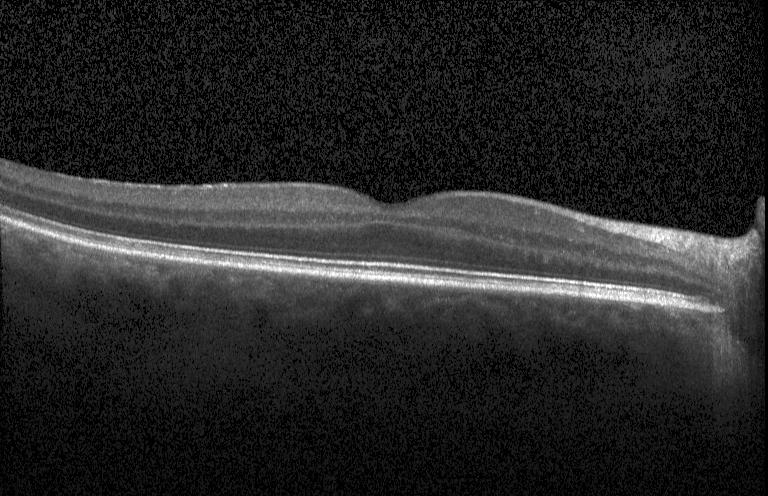
SD-OCT, instrument: Heidelberg Spectralis, OCT B-scan, horizontal scan through the fovea. Impression: no CNV, DME, or drusen.